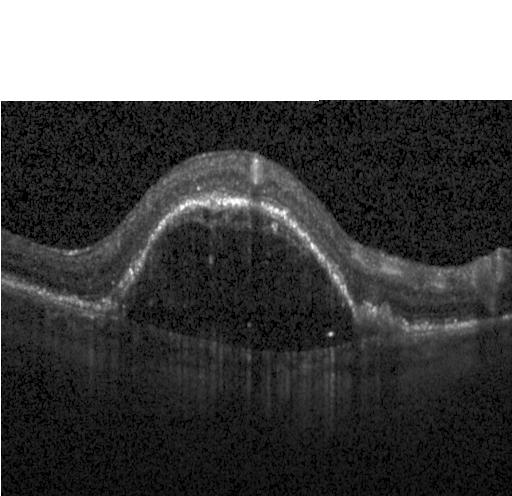

This B-scan demonstrates choroidal neovascularization.